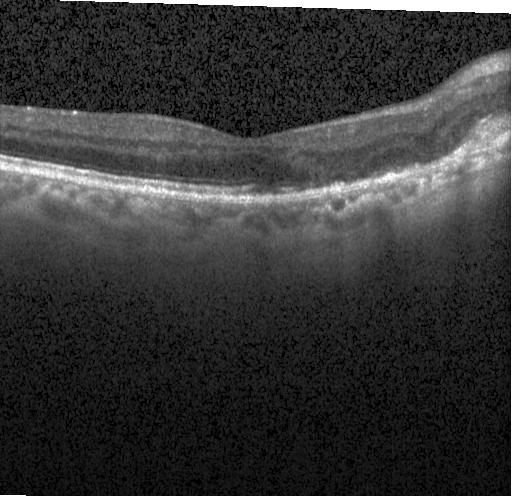
OCT line scan — Assessment: a choroidal neovascular membrane.